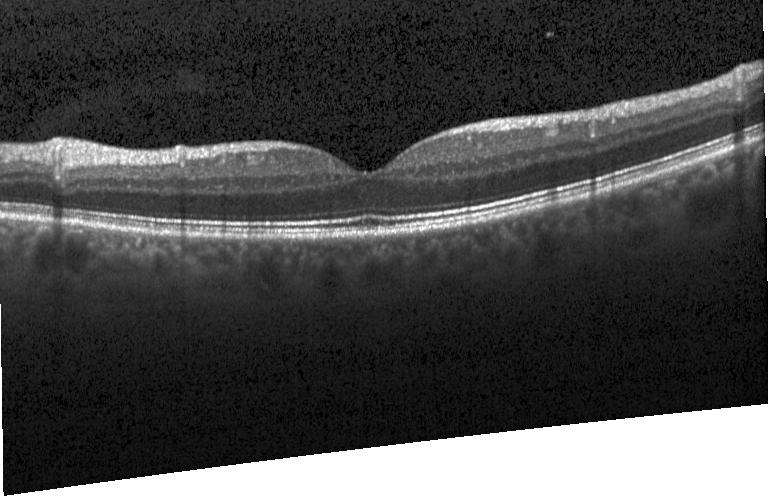

SD-OCT, macular scan, optical coherence tomography B-scan — Diagnosis: neither choroidal neovascularization, diabetic macular edema, nor drusen.